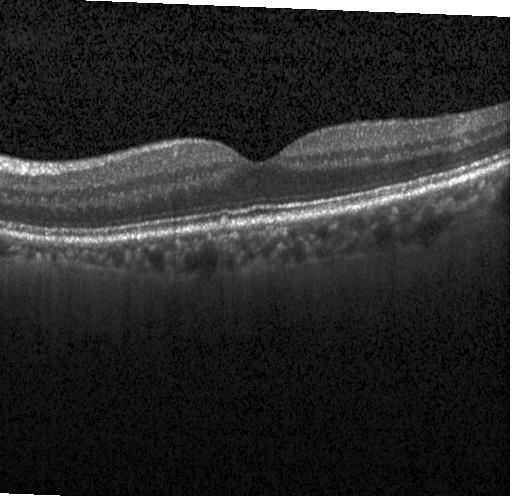
OCT line scan, instrument: Heidelberg Spectralis.
Impression: neither choroidal neovascularization, diabetic macular edema, nor drusen.